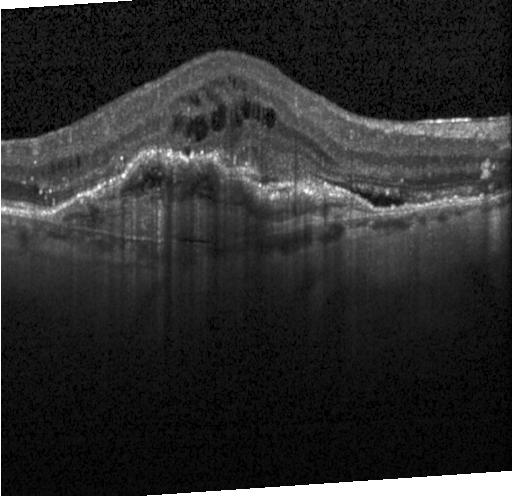

Optical coherence tomography B-scan.
Finding: a choroidal neovascular membrane.